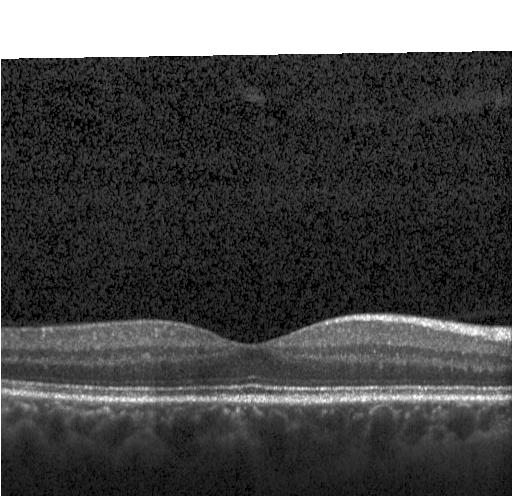

Macular OCT demonstrating neither choroidal neovascularization, diabetic macular edema, nor drusen.